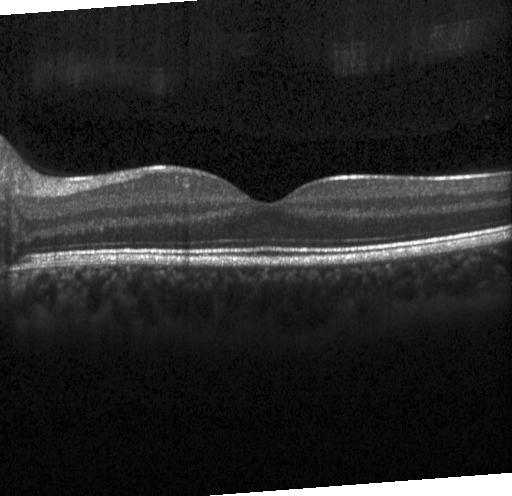
Retinal OCT cross-section — Impression: no choroidal neovascularization, diabetic macular edema, or drusen.